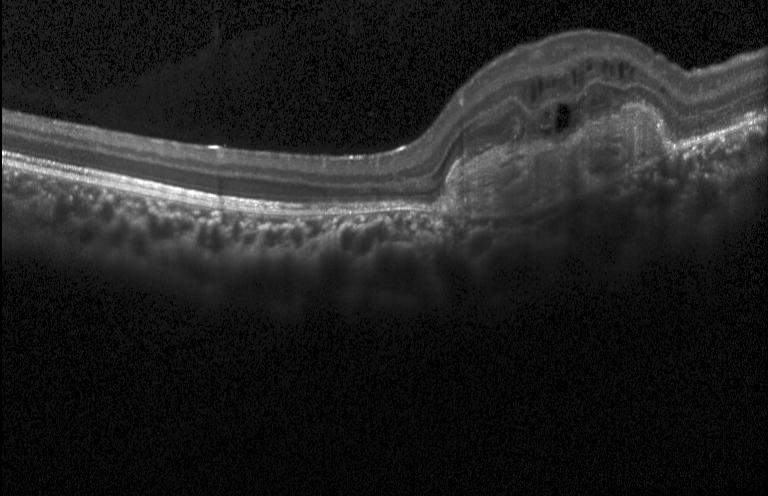

Optical coherence tomography scan, fovea-centered
This B-scan demonstrates choroidal neovascularization (CNV).